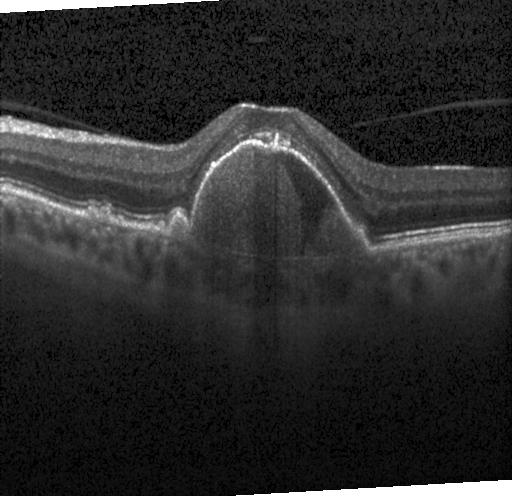
Macular OCT: a choroidal neovascular membrane.